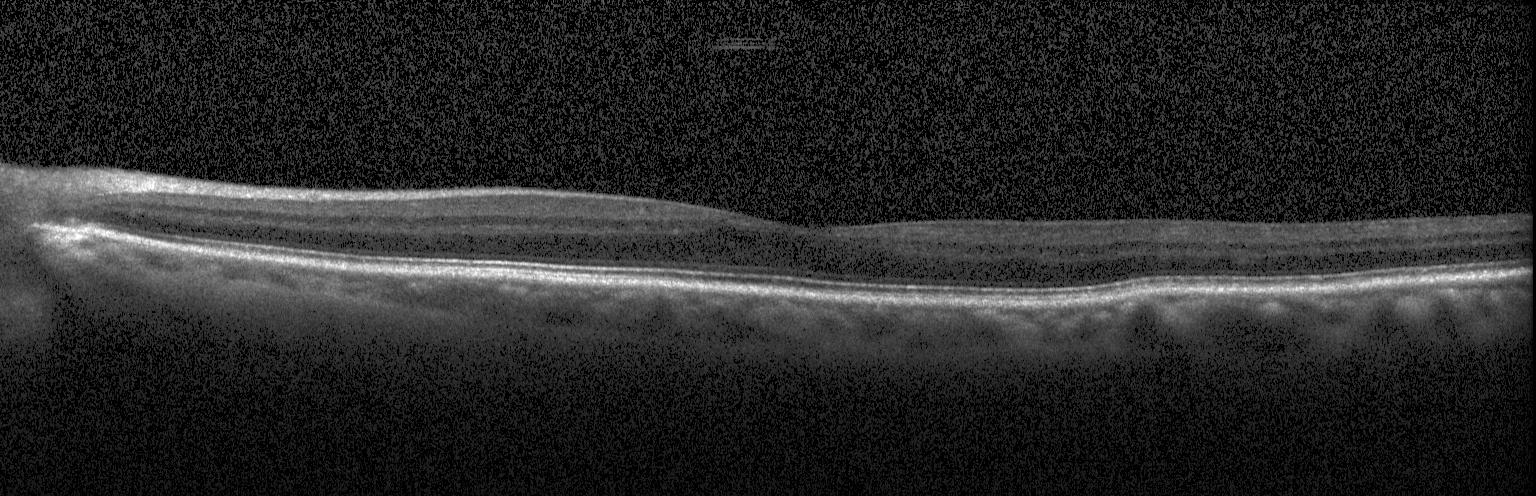

Retinal OCT B-scan. Instrument: Heidelberg Spectralis. SD-OCT. Horizontal scan through the fovea
No CNV, DME, or drusen.